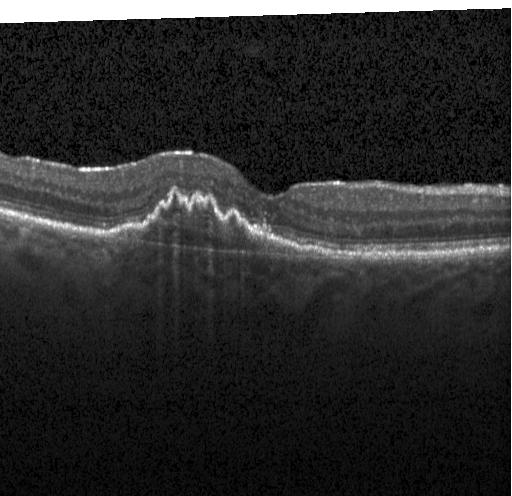
Retinal OCT B-scan, through the macula — A choroidal neovascular membrane.